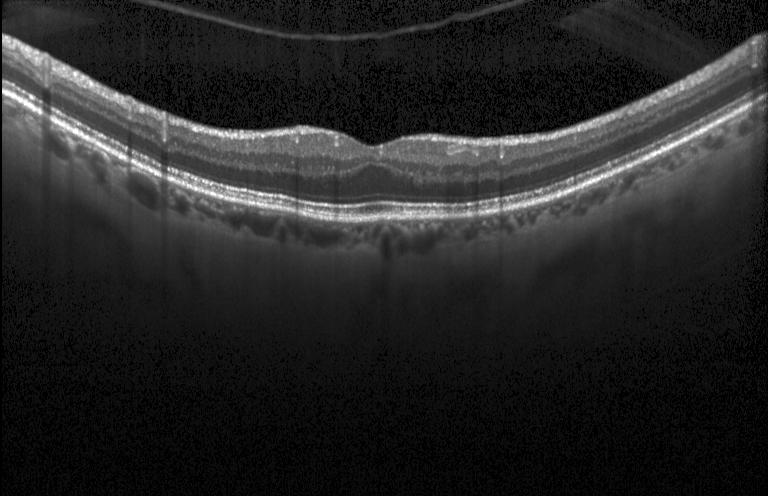 Retinal OCT cross-section. Assessment: no evidence of choroidal neovascularization, diabetic macular edema, or drusen.